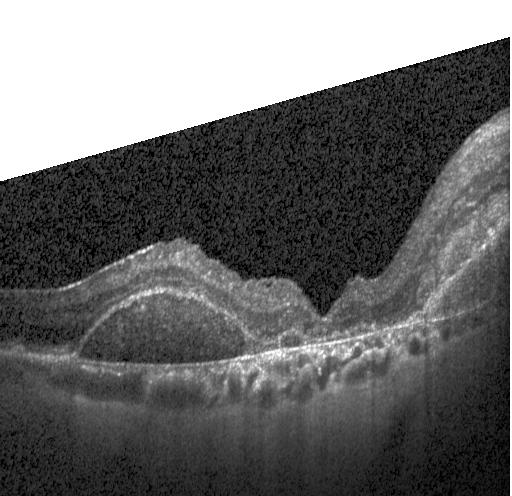
OCT line scan, spectral-domain OCT, acquired on a Heidelberg Spectralis, horizontal scan through the fovea
Impression: choroidal neovascularization (CNV).